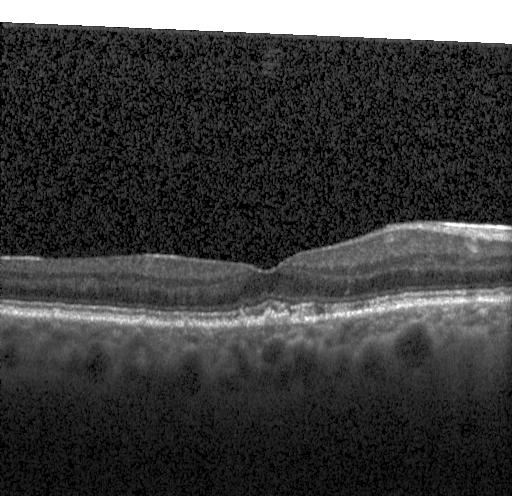

Instrument: Heidelberg Spectralis, spectral-domain OCT, optical coherence tomography B-scan.
Diagnosis: sub-RPE drusenoid deposits.